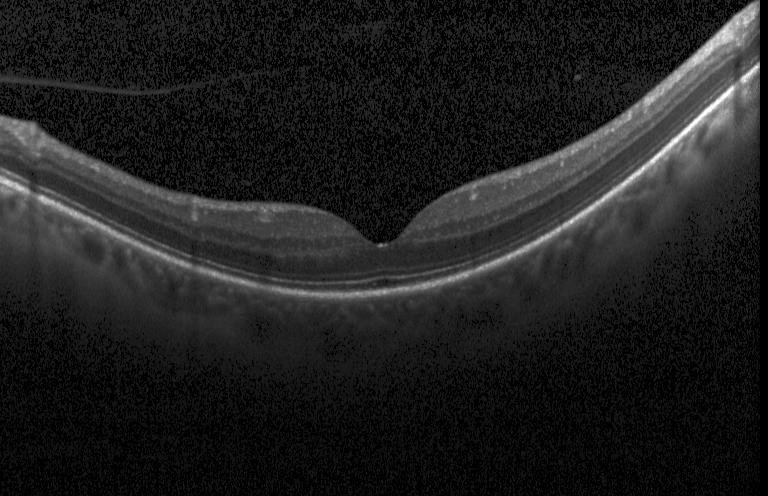 The scan shows no evidence of CNV, DME, or drusen.